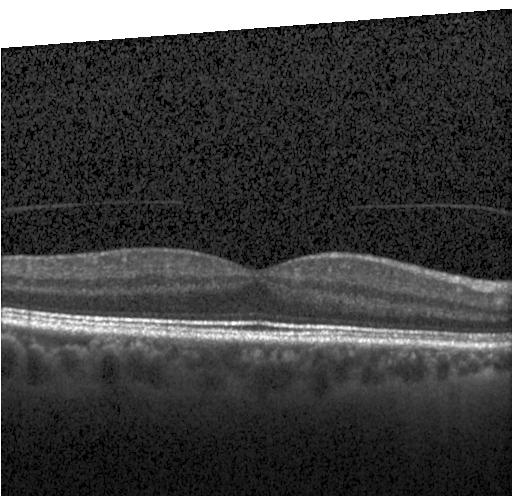
Retinal OCT B-scan. Impression: no CNV, no DME, and no drusen.